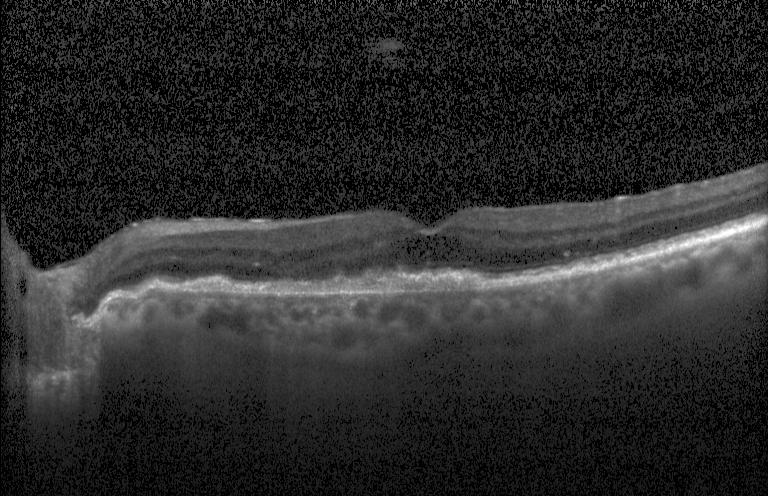

Optical coherence tomography scan. Spectral-domain OCT. Instrument: Heidelberg Spectralis. Horizontal scan through the fovea. Impression: a choroidal neovascular membrane.